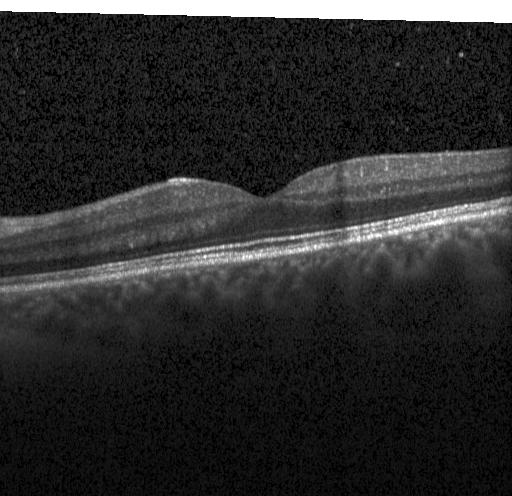

Heidelberg Spectralis, OCT line scan, horizontal scan through the fovea, spectral-domain OCT
OCT finding: no CNV, DME, or drusen.